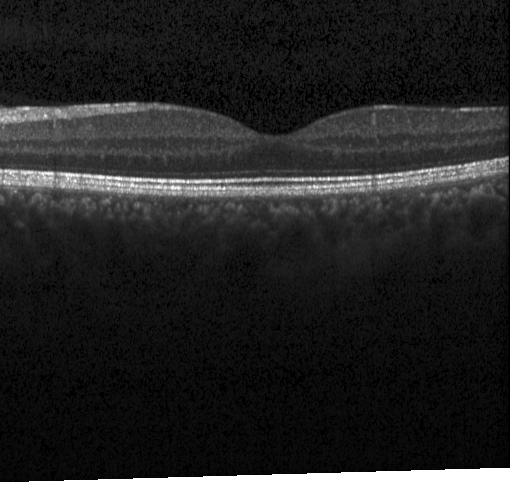 Optical coherence tomography scan — Impression: no choroidal neovascularization, no diabetic macular edema, and no drusen.